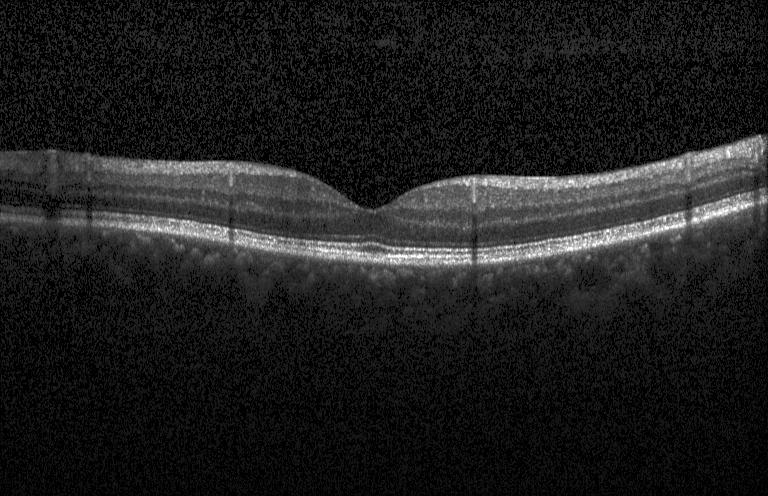 Diagnosis: no choroidal neovascularization, no diabetic macular edema, and no drusen.